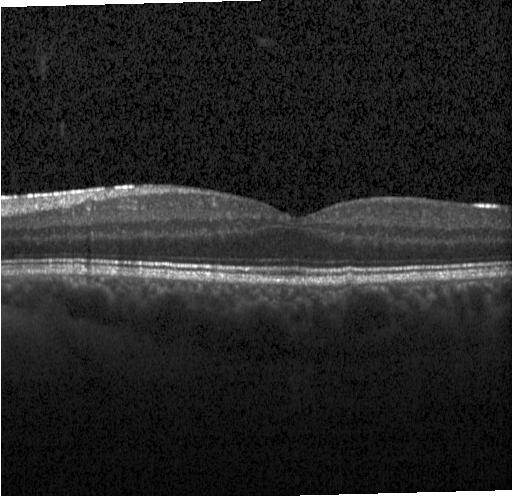
Impression: no evidence of choroidal neovascularization, diabetic macular edema, or drusen.